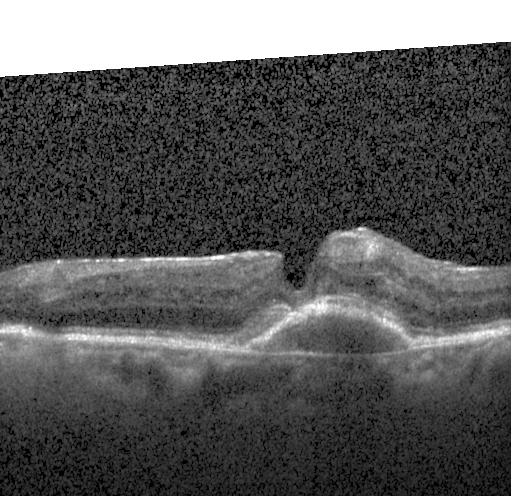
Finding: choroidal neovascularization (CNV).